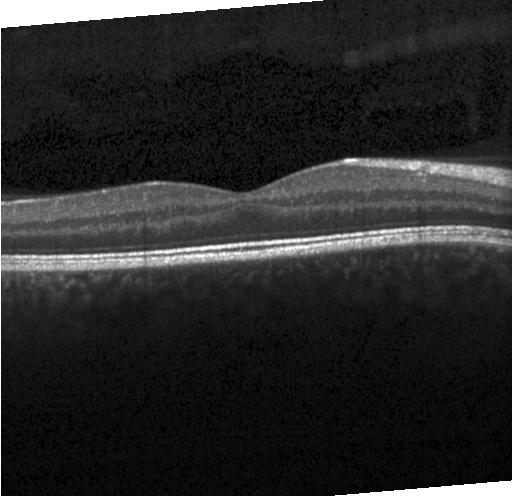
Spectral-domain optical coherence tomography. Heidelberg Spectralis. Horizontal scan through the fovea. Retinal OCT B-scan
The scan shows no evidence of choroidal neovascularization, diabetic macular edema, or drusen.